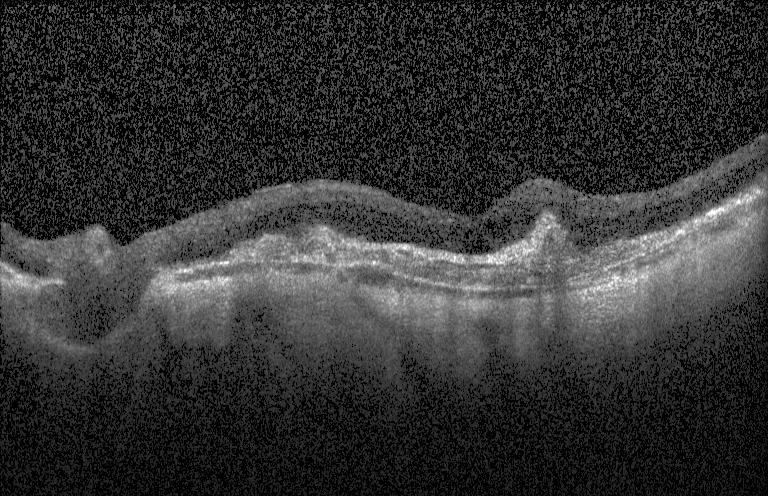
Optical coherence tomography scan. SD-OCT. Heidelberg Spectralis OCT system. Fovea-centered. The scan shows a choroidal neovascular membrane.